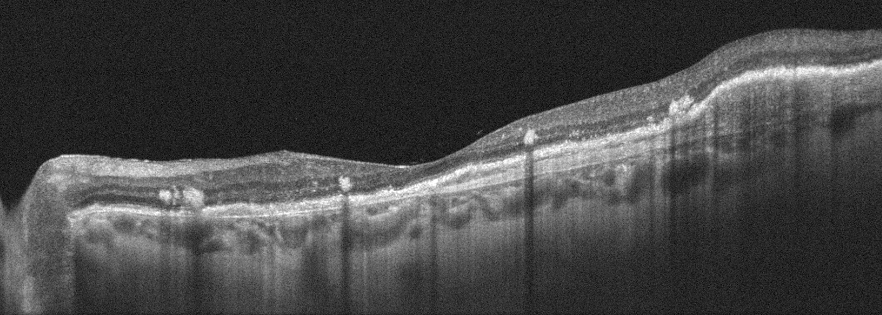 Left eye. Retinal OCT cross-section. Fovea-centered. Acquired on an Optovue Avanti RTVue XR — Finding: age-related macular degeneration (AMD).